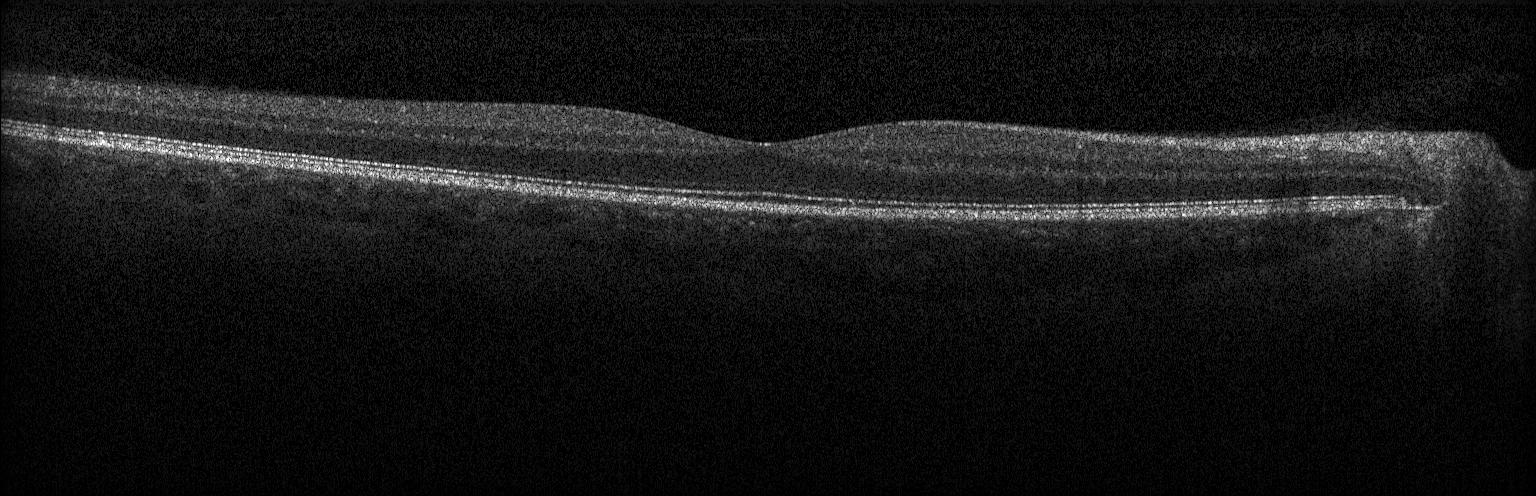 Instrument: Heidelberg Spectralis · spectral-domain OCT · retinal OCT B-scan · through the macula. Finding: no evidence of choroidal neovascularization, diabetic macular edema, or drusen.